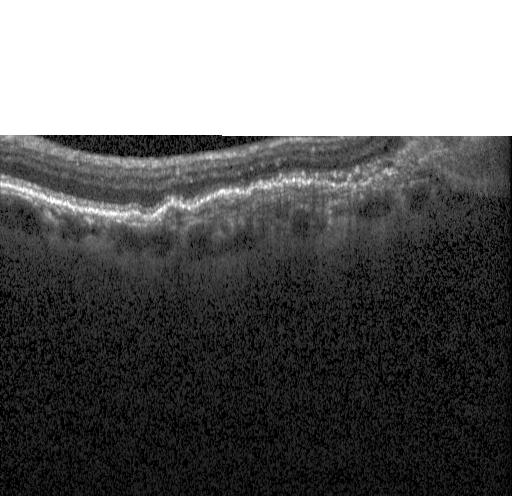 Spectral-domain OCT B-scan: CNV.